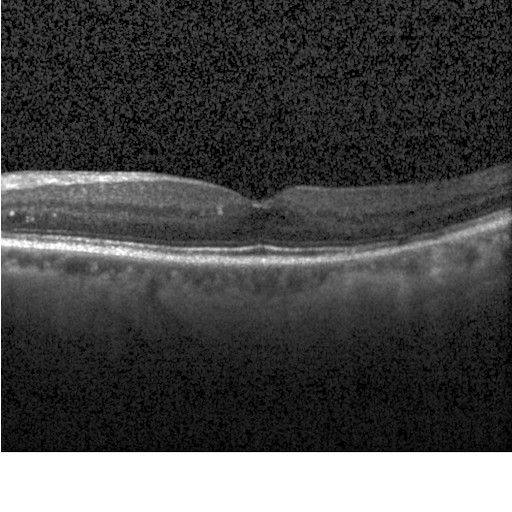

Optical coherence tomography scan.
Macular OCT: DME.